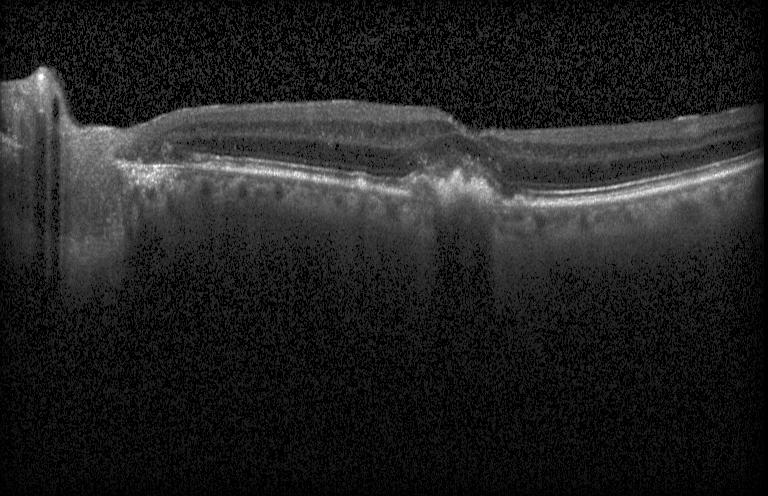 Acquired on a Heidelberg Spectralis · OCT B-scan — Impression: choroidal neovascularization.